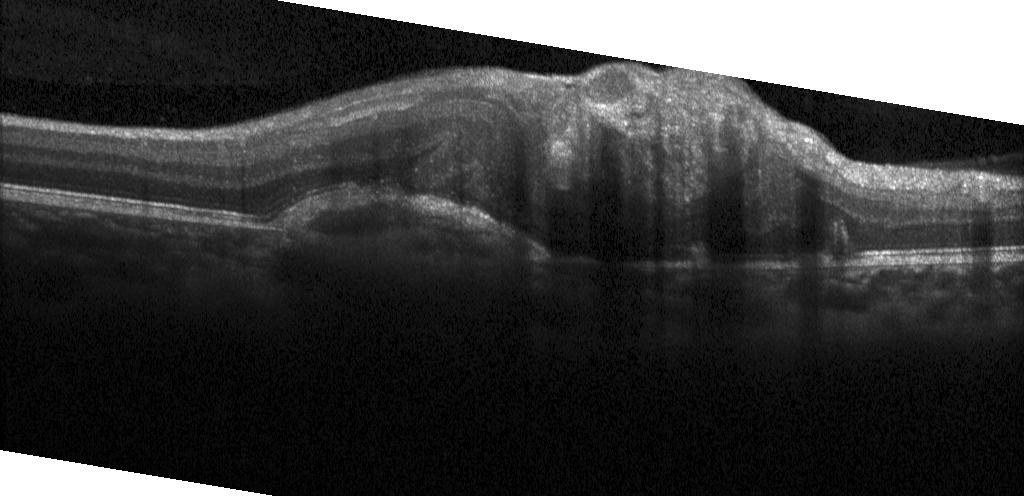 OCT B-scan showing CNV.